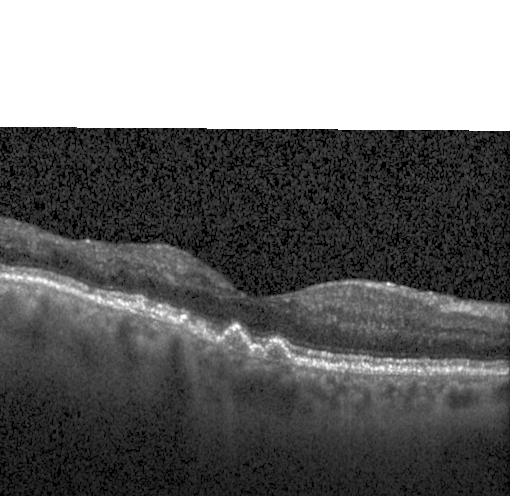

Acquired on a Heidelberg Spectralis; OCT B-scan; SD-OCT. Finding: drusen.